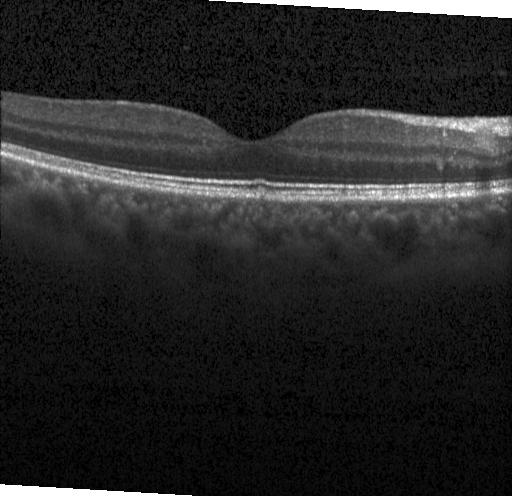

Diagnosis: neither CNV, DME, nor drusen.